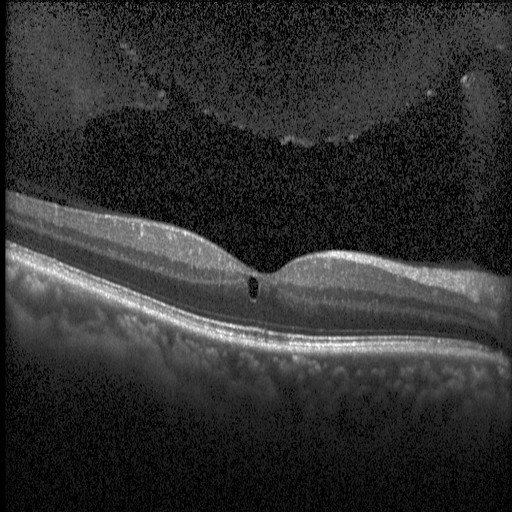 OCT finding: DME.